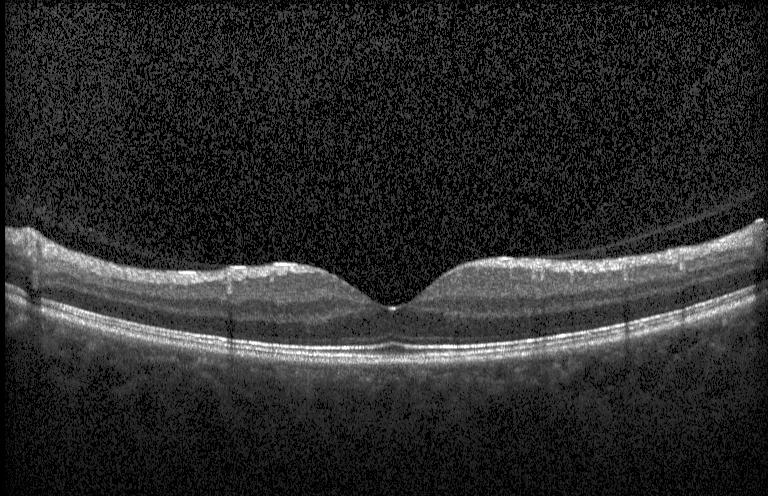
Optical coherence tomography scan; Heidelberg Spectralis; SD-OCT; fovea-centered. Impression: no CNV, DME, or drusen.